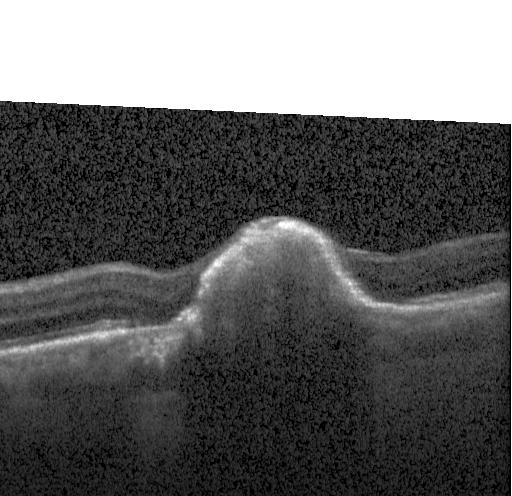
Retinal OCT B-scan, spectral-domain OCT, Heidelberg Spectralis OCT system. Diagnosis: choroidal neovascularization (CNV).